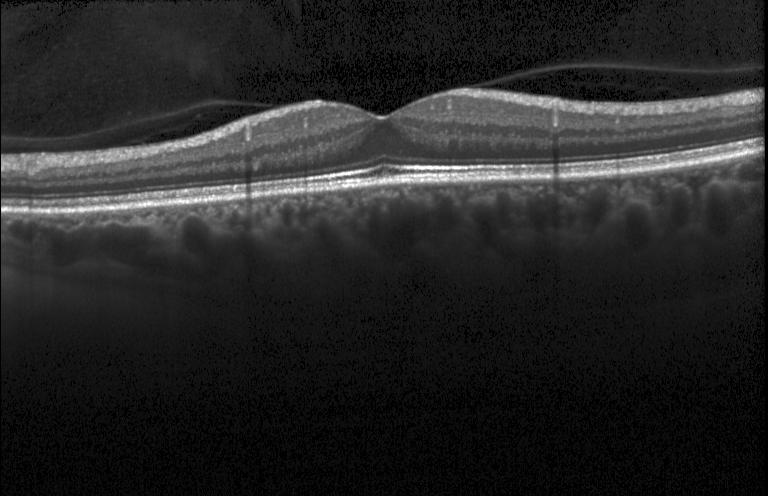

SD-OCT · retinal OCT cross-section — This B-scan demonstrates no choroidal neovascularization, diabetic macular edema, or drusen.